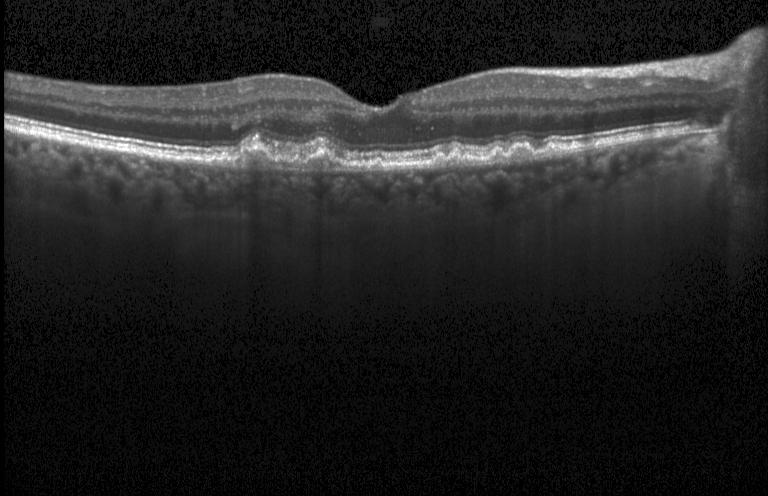
Diagnosis: multiple drusen.